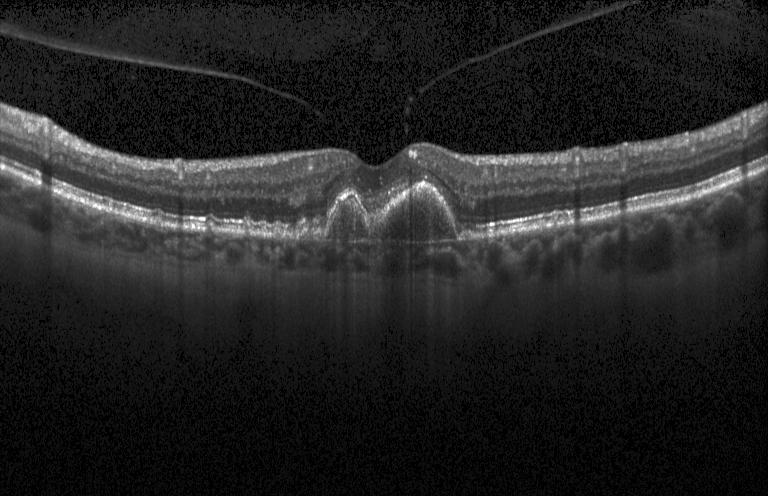
Fovea-centered. OCT line scan. Acquired on a Heidelberg Spectralis. SD-OCT.
A choroidal neovascular membrane.